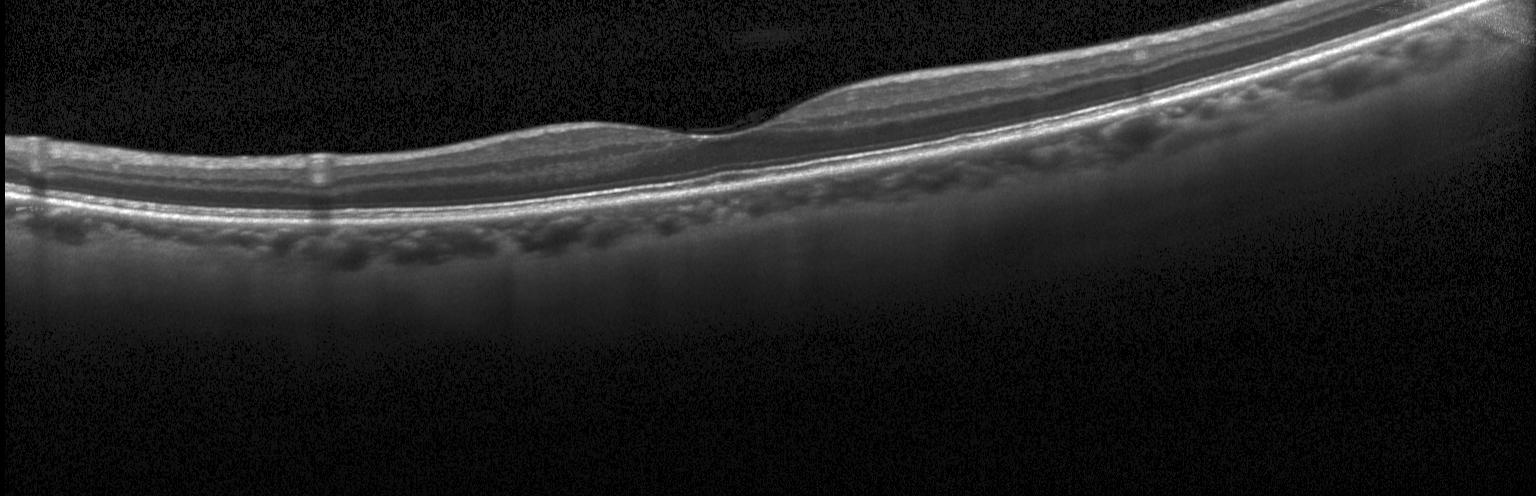 Dx: no evidence of choroidal neovascularization, diabetic macular edema, or drusen.